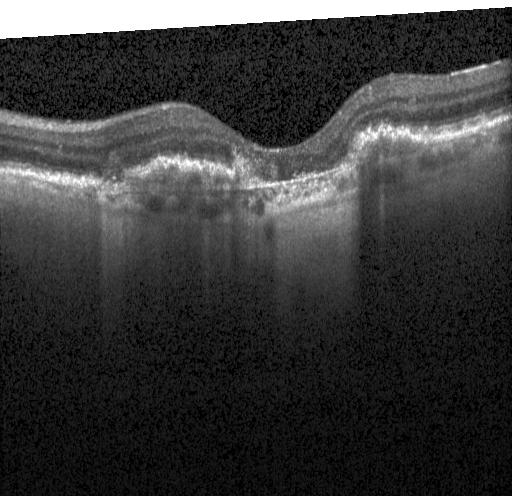
Macular OCT demonstrating a choroidal neovascular membrane.